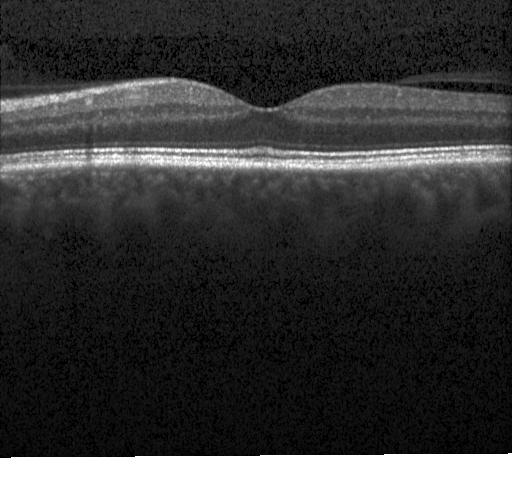

Retinal OCT B-scan — Finding: no evidence of choroidal neovascularization, diabetic macular edema, or drusen.